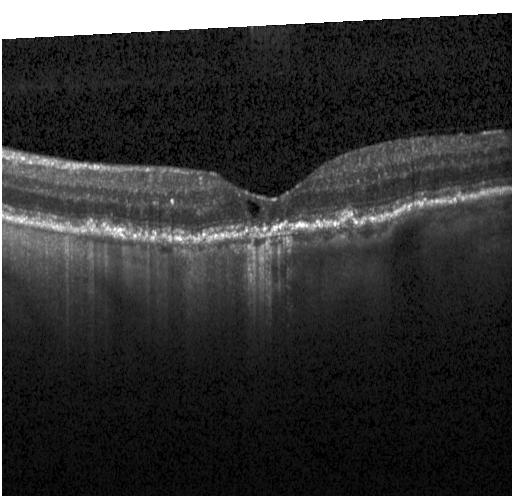
Dx: a choroidal neovascular membrane.